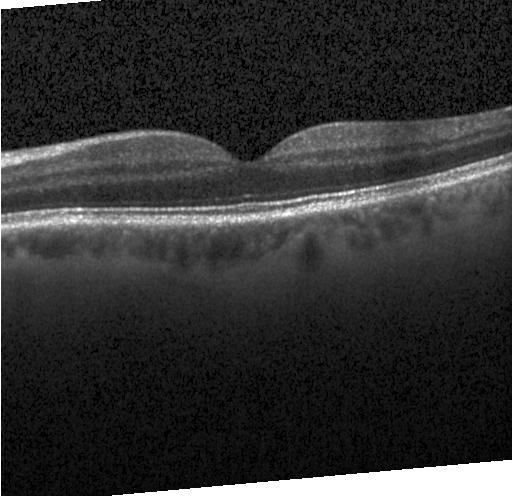

Optical coherence tomography scan · Heidelberg Spectralis · fovea-centered. This B-scan demonstrates no evidence of choroidal neovascularization, diabetic macular edema, or drusen.